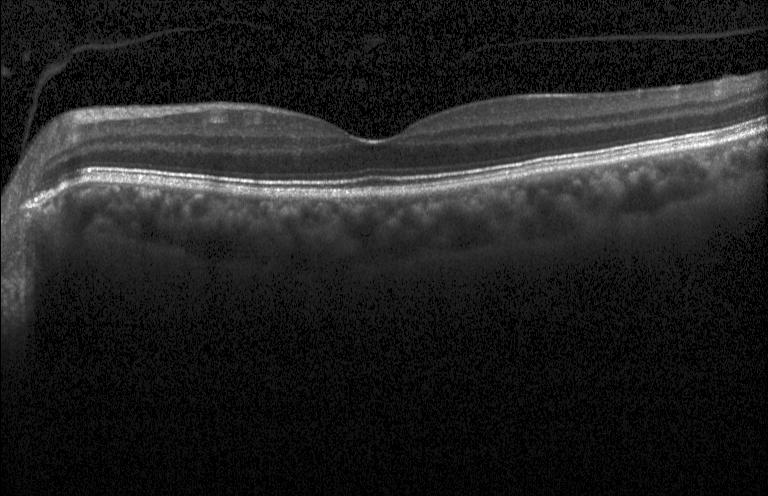
This B-scan demonstrates no evidence of choroidal neovascularization, diabetic macular edema, or drusen.